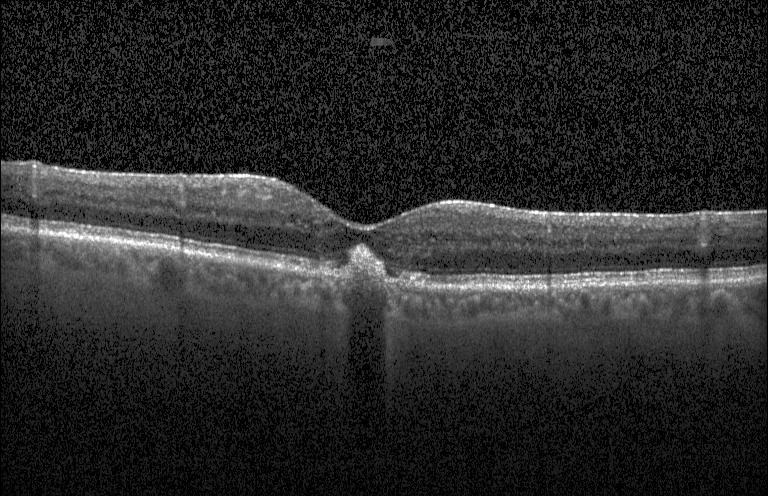
Acquired on a Heidelberg Spectralis · fovea-centered · retinal OCT cross-section
Dx: CNV.